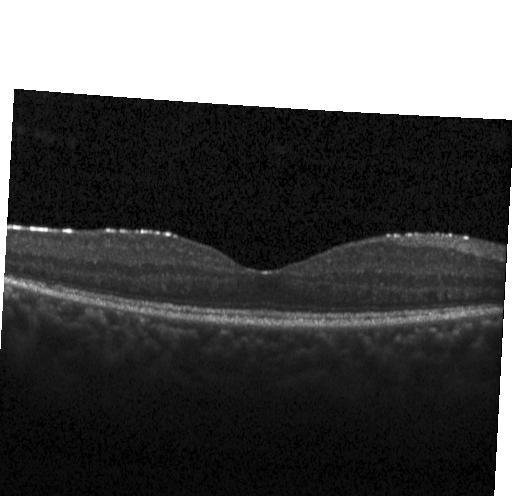

Acquired on a Heidelberg Spectralis, retinal OCT cross-section — Finding: no evidence of CNV, DME, or drusen.